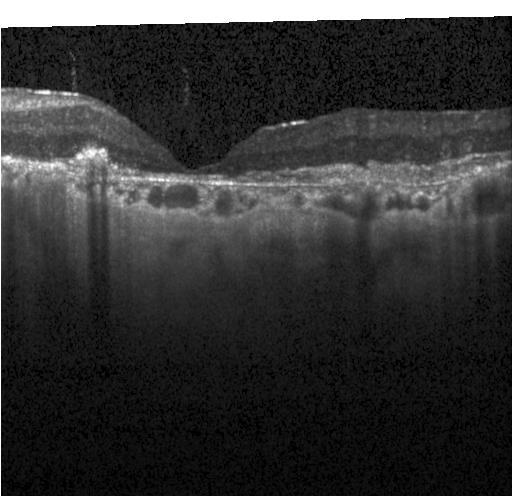 Fovea-centered · retinal OCT B-scan · spectral-domain optical coherence tomography · Heidelberg Spectralis OCT system. Diagnosis: CNV.